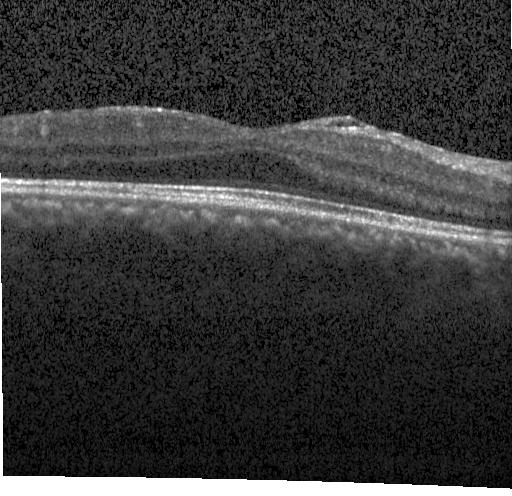
Centered on the fovea, spectral-domain optical coherence tomography, retinal OCT cross-section. Diagnosis: no CNV, no DME, and no drusen.